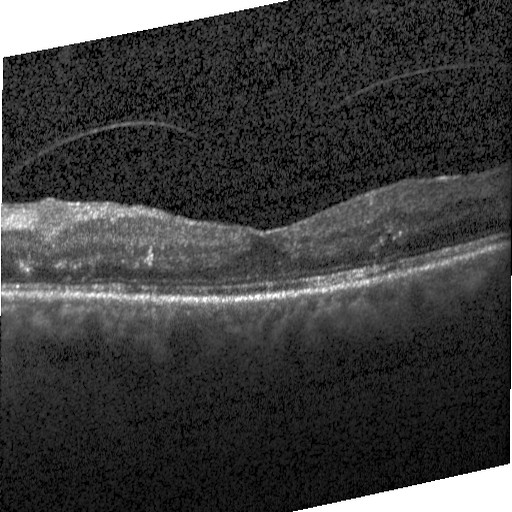
Heidelberg Spectralis OCT system. Optical coherence tomography B-scan. Fovea-centered. Spectral-domain optical coherence tomography — This B-scan demonstrates diabetic macular edema.